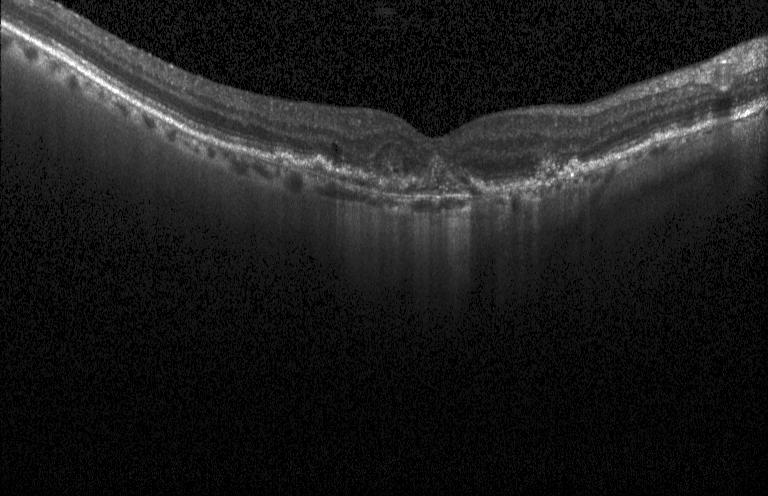

Spectral-domain optical coherence tomography. OCT B-scan. Centered on the fovea. Heidelberg Spectralis.
A choroidal neovascular membrane.